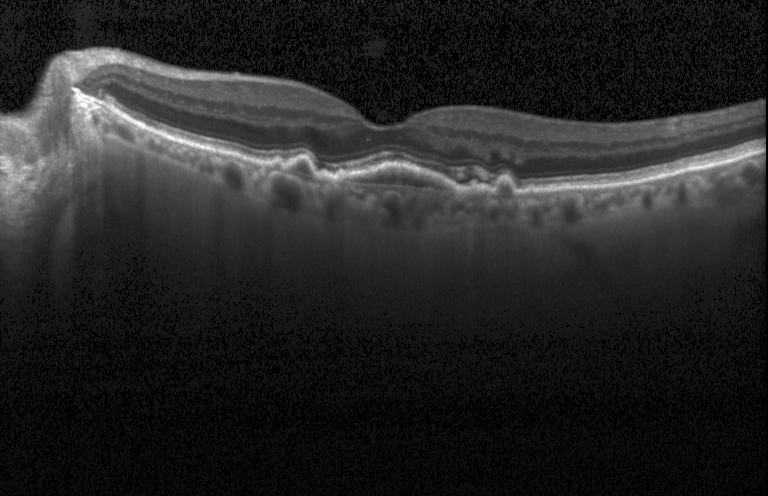

Macular OCT demonstrating choroidal neovascularization (CNV).